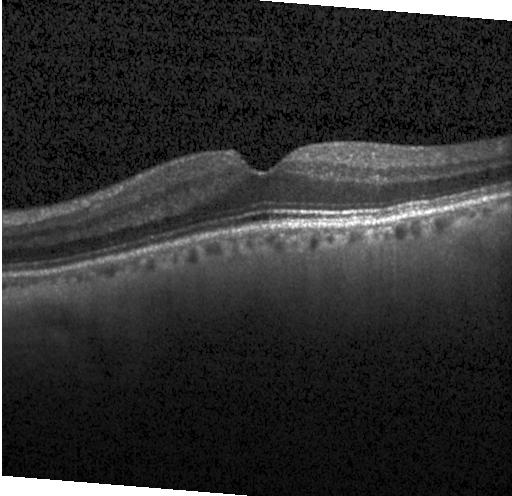

Impression: no evidence of CNV, DME, or drusen.